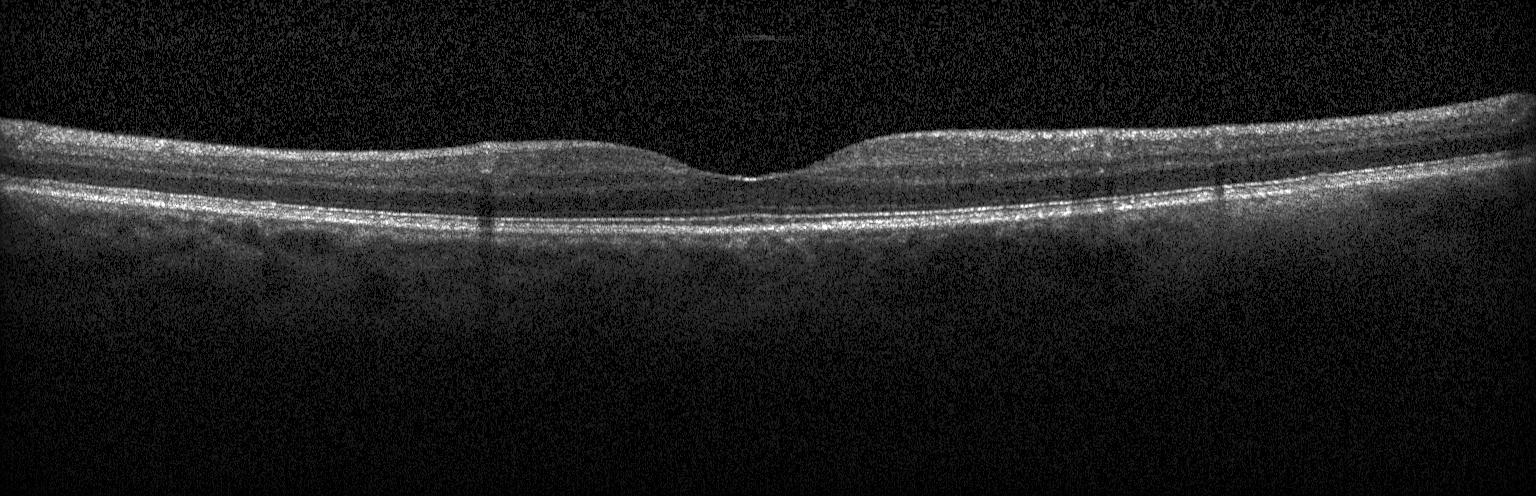 Macular OCT demonstrating neither choroidal neovascularization, diabetic macular edema, nor drusen.